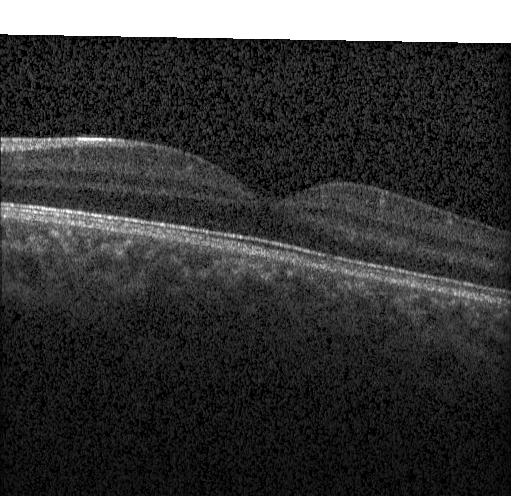
Optical coherence tomography scan. Heidelberg Spectralis. Spectral-domain optical coherence tomography.
Diagnosis: no evidence of CNV, DME, or drusen.